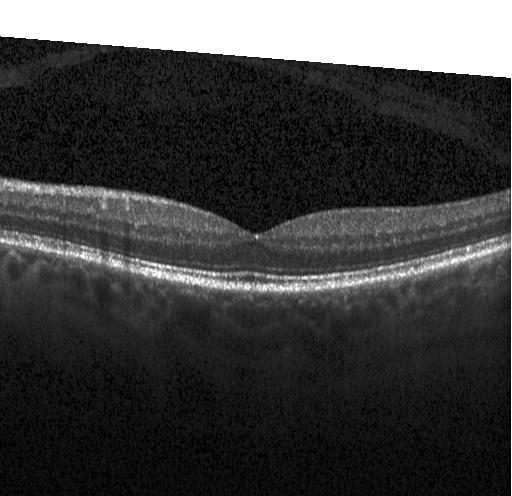

Finding: no evidence of CNV, DME, or drusen.